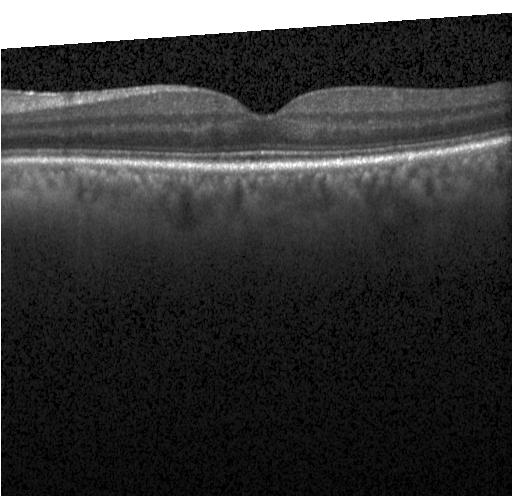

Macular OCT: neither CNV, DME, nor drusen.